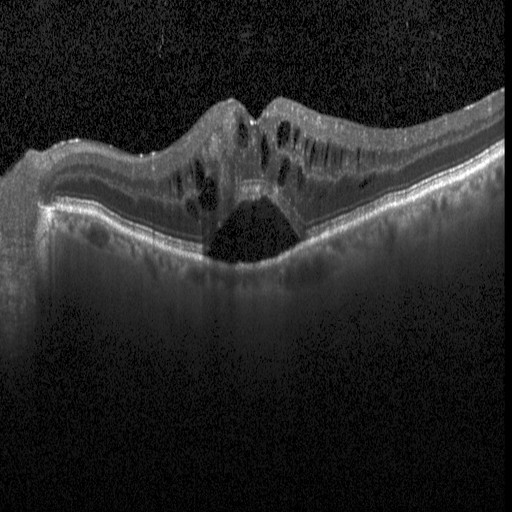
Heidelberg Spectralis OCT system · optical coherence tomography scan · SD-OCT · horizontal scan through the fovea.
Impression: diabetic macular edema.